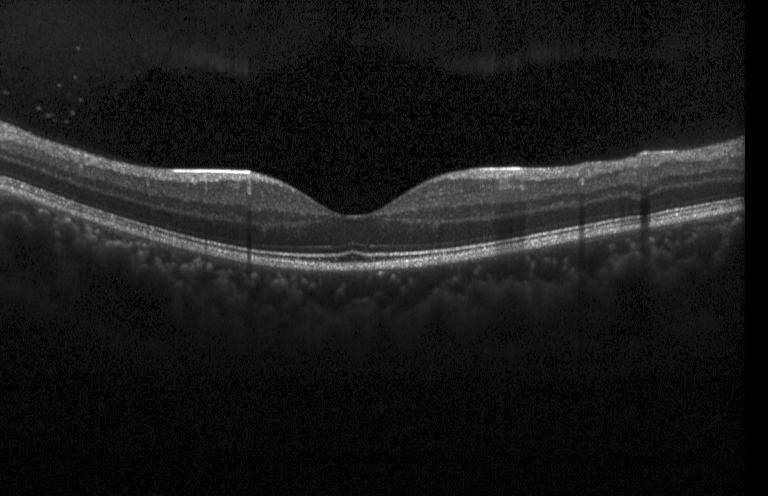

Fovea-centered · retinal OCT cross-section · instrument: Heidelberg Spectralis · spectral-domain optical coherence tomography. This B-scan demonstrates no choroidal neovascularization, diabetic macular edema, or drusen.